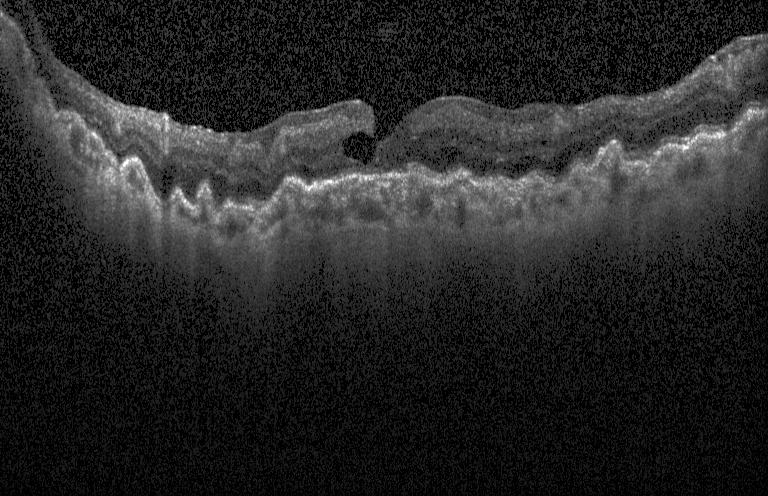 OCT B-scan, SD-OCT, instrument: Heidelberg Spectralis, centered on the fovea. This B-scan demonstrates choroidal neovascularization.